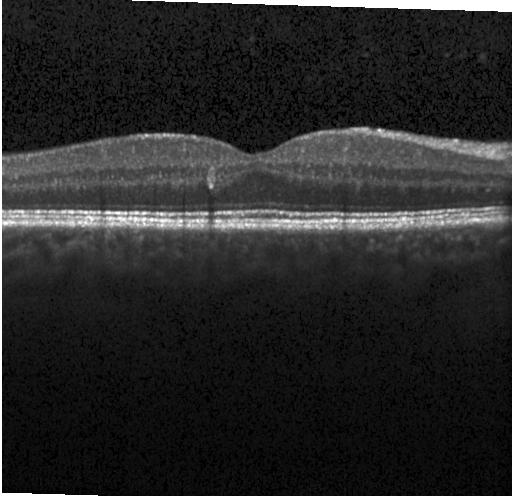
OCT scan showing no choroidal neovascularization, diabetic macular edema, or drusen.